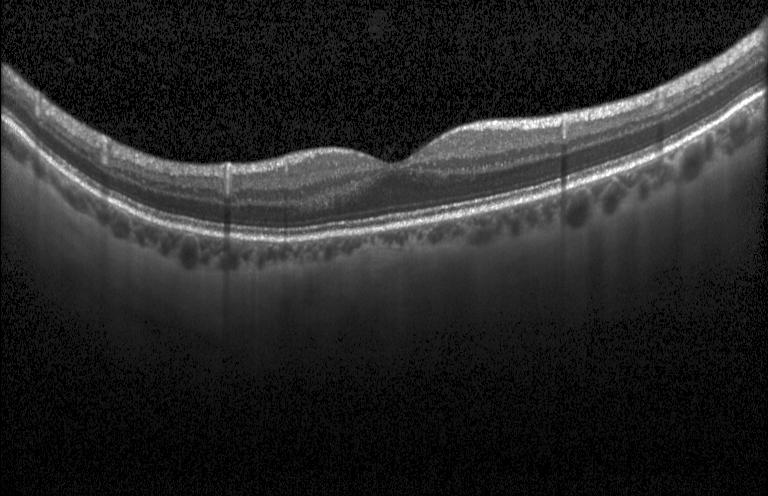
Instrument: Heidelberg Spectralis. Optical coherence tomography B-scan. SD-OCT.
This B-scan demonstrates no evidence of CNV, DME, or drusen.